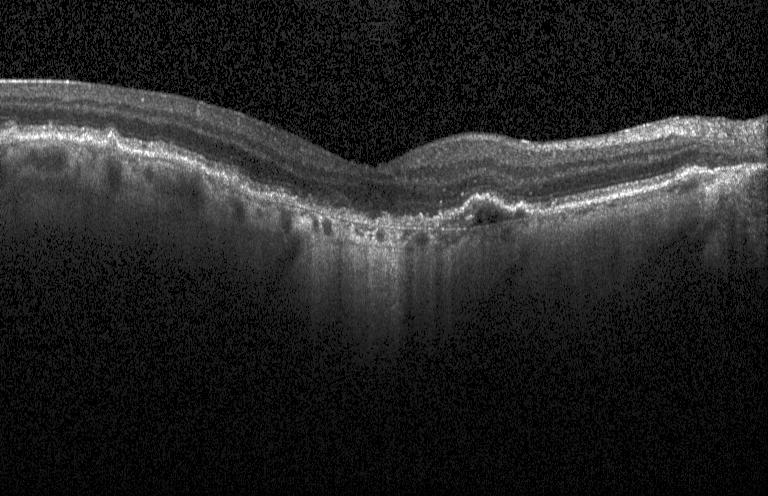
Optical coherence tomography scan — Diagnosis: a choroidal neovascular membrane.